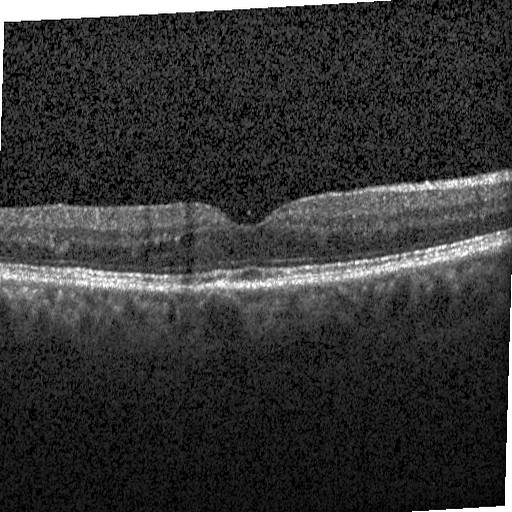

Impression: DME.